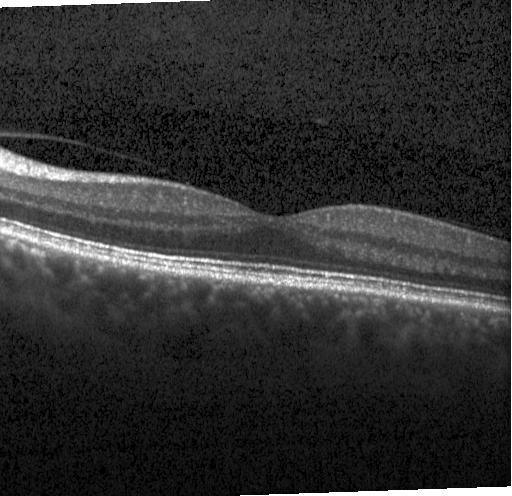
OCT scan showing no evidence of choroidal neovascularization, diabetic macular edema, or drusen.